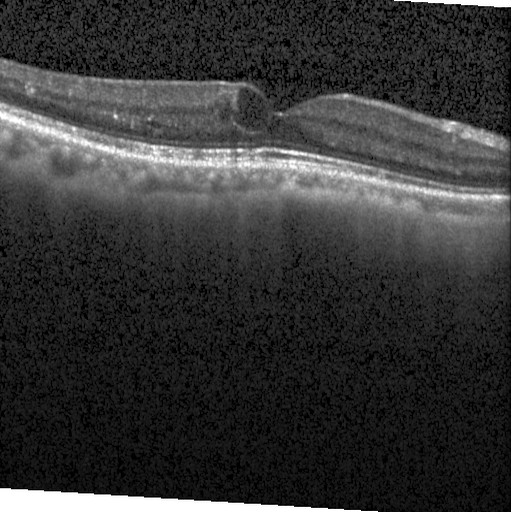

Acquired on a Heidelberg Spectralis · fovea-centered · spectral-domain optical coherence tomography · retinal OCT B-scan.
Diabetic macular edema.